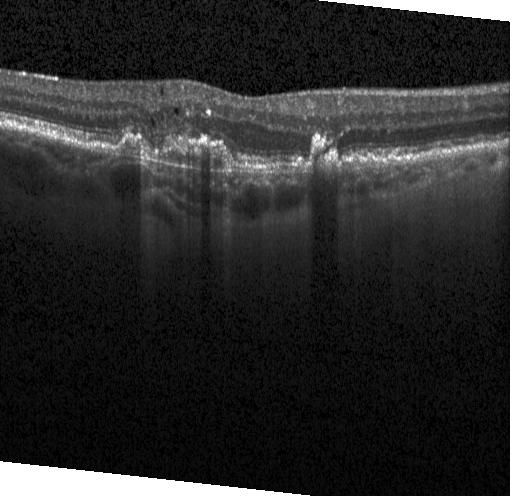

Impression: a choroidal neovascular membrane.